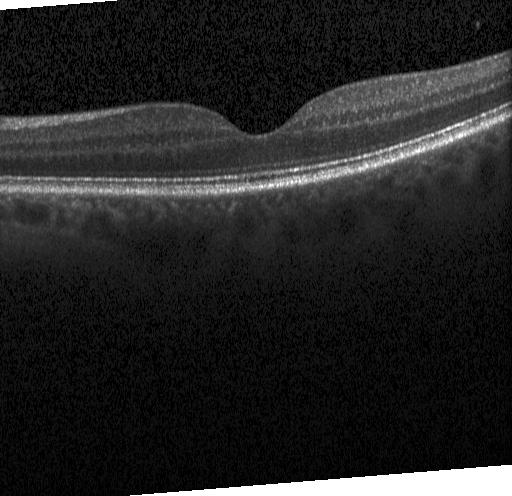

Acquired on a Heidelberg Spectralis, OCT B-scan — Diagnosis: neither choroidal neovascularization, diabetic macular edema, nor drusen.